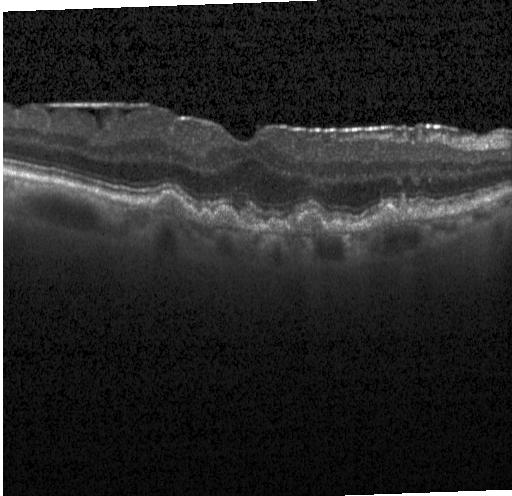

Retinal OCT cross-section. OCT finding: multiple drusen.